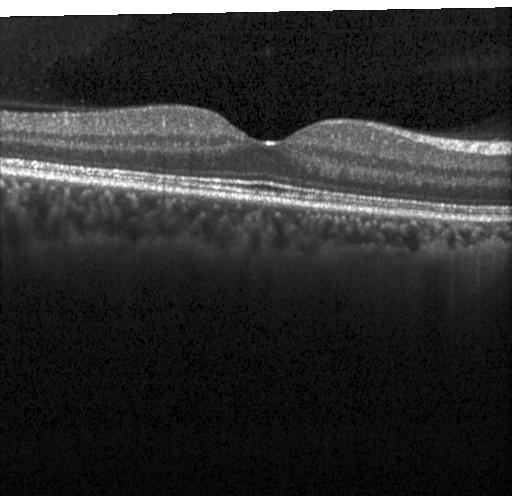

Macular OCT demonstrating no evidence of CNV, DME, or drusen.